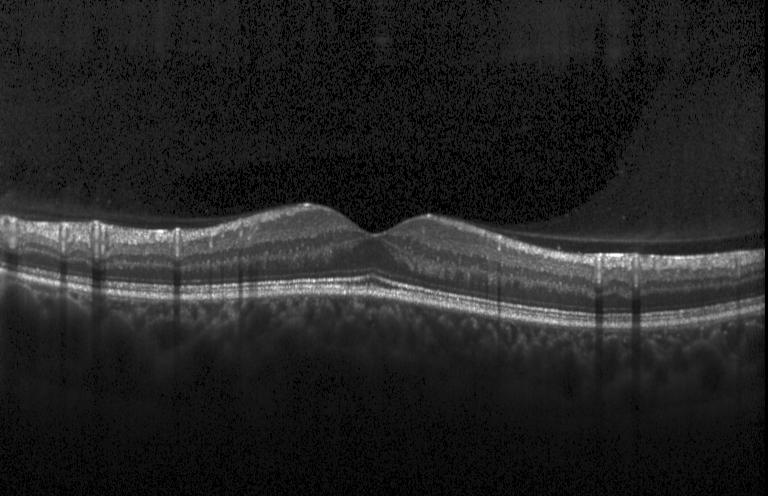 OCT line scan · SD-OCT.
Impression: no choroidal neovascularization, diabetic macular edema, or drusen.